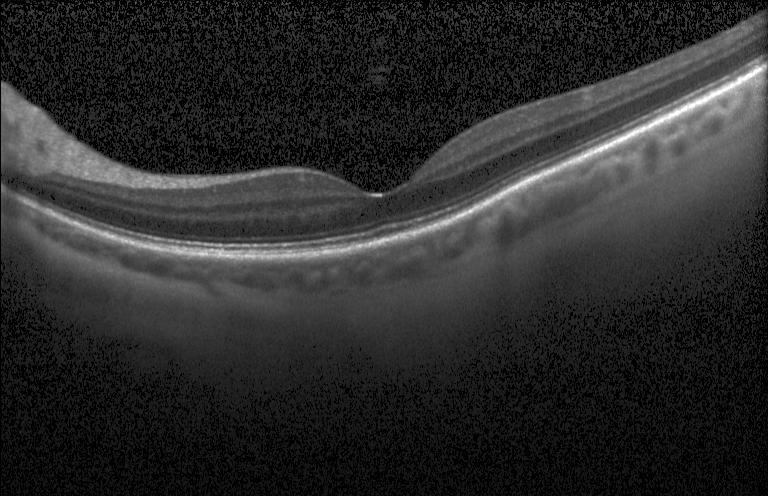 Retinal OCT B-scan · spectral-domain OCT.
Impression: neither choroidal neovascularization, diabetic macular edema, nor drusen.